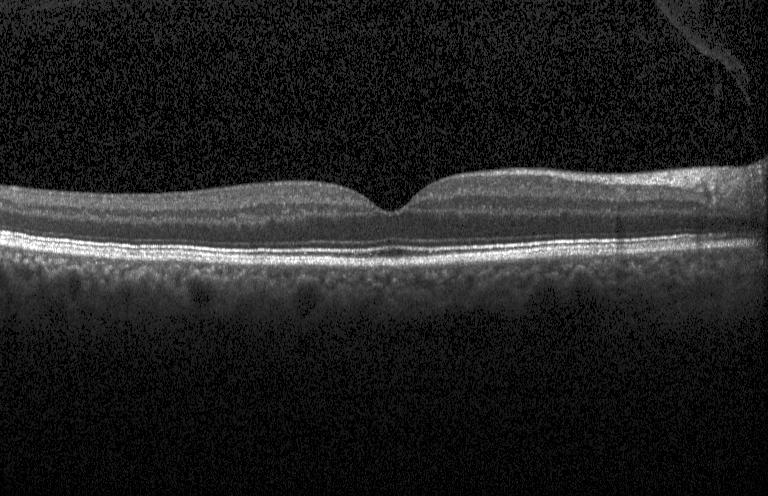 Dx: no evidence of choroidal neovascularization, diabetic macular edema, or drusen.